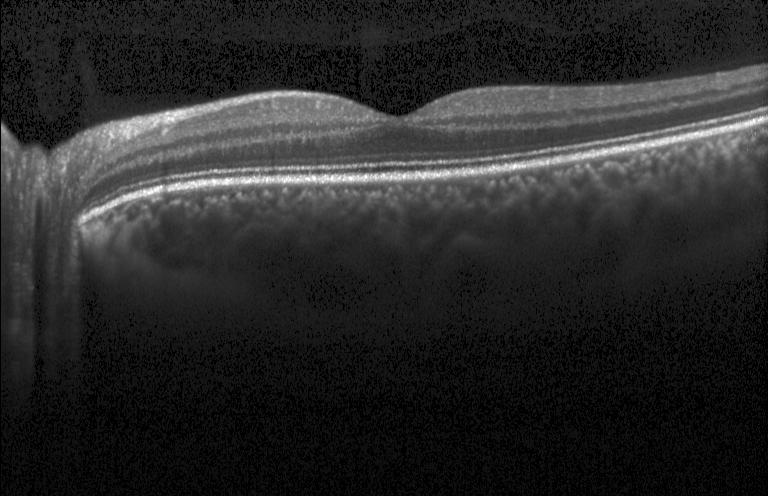 Heidelberg Spectralis OCT system, retinal OCT cross-section, through the macula.
Diagnosis: no evidence of CNV, DME, or drusen.